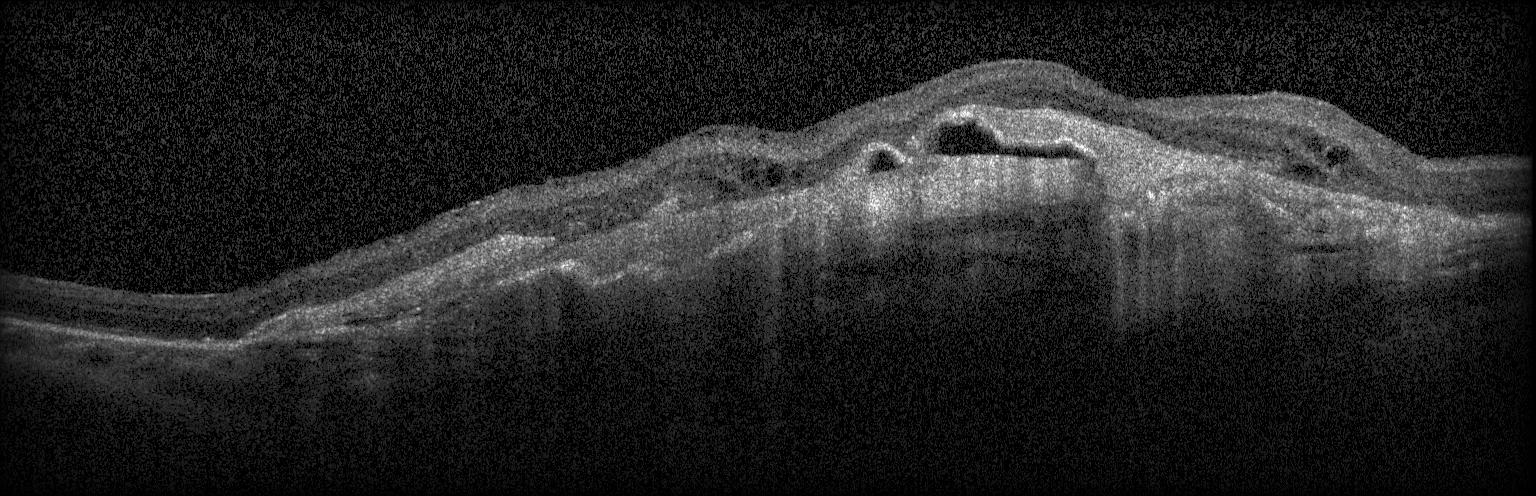

Heidelberg Spectralis, retinal OCT cross-section, spectral-domain optical coherence tomography
This B-scan demonstrates a choroidal neovascular membrane.